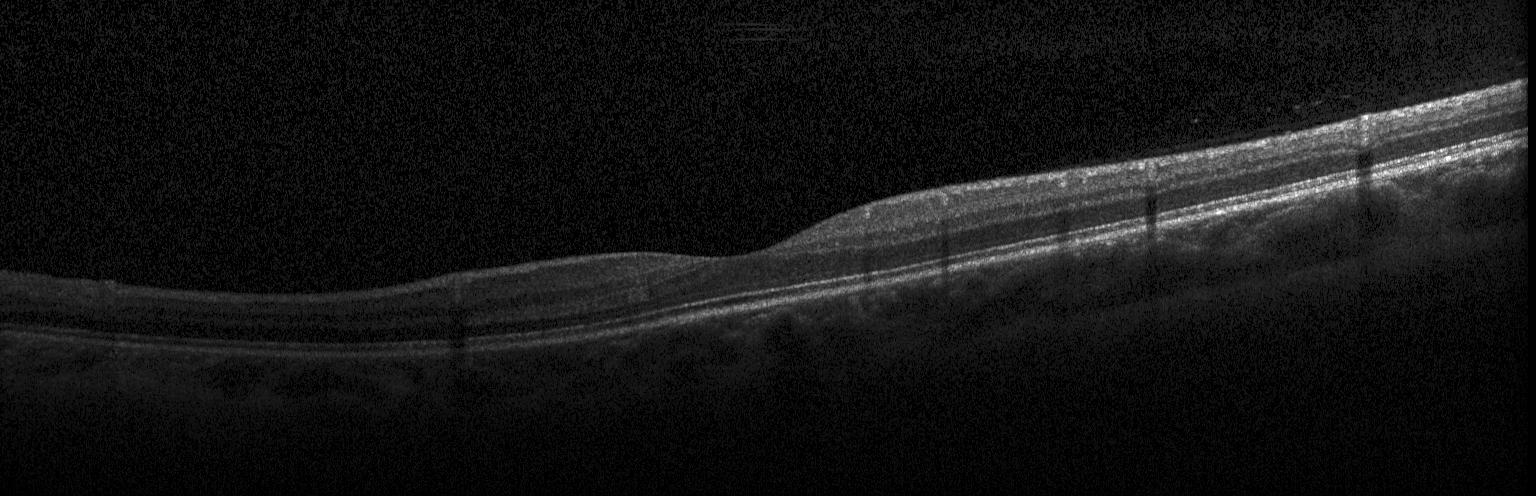 Neither choroidal neovascularization, diabetic macular edema, nor drusen.